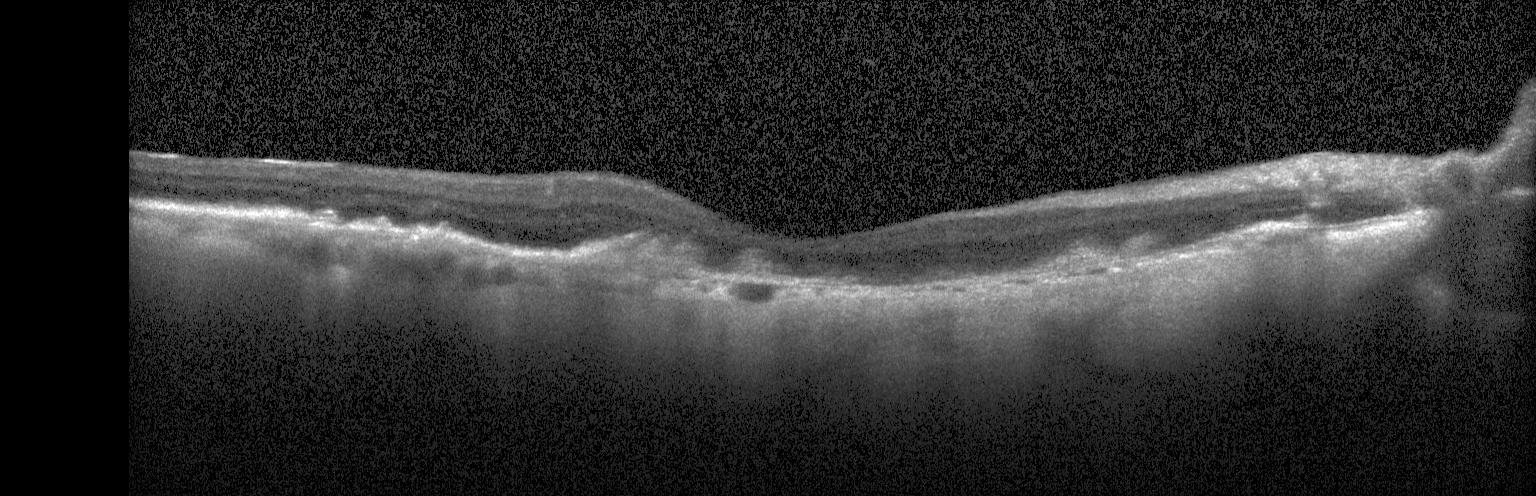

OCT B-scan showing a choroidal neovascular membrane.